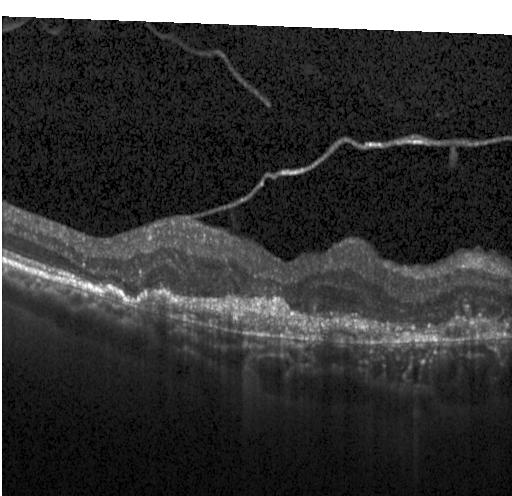

Finding: CNV.